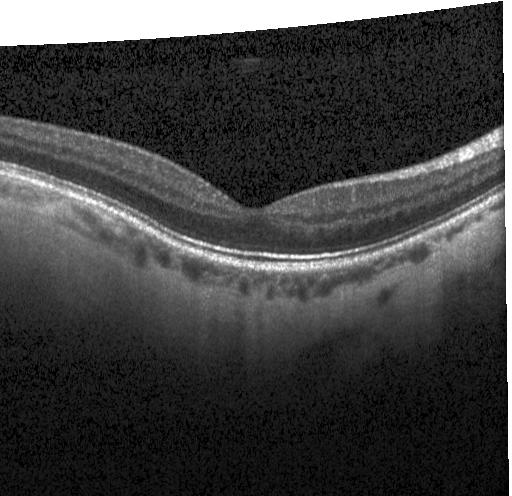 Spectral-domain OCT B-scan: neither CNV, DME, nor drusen.